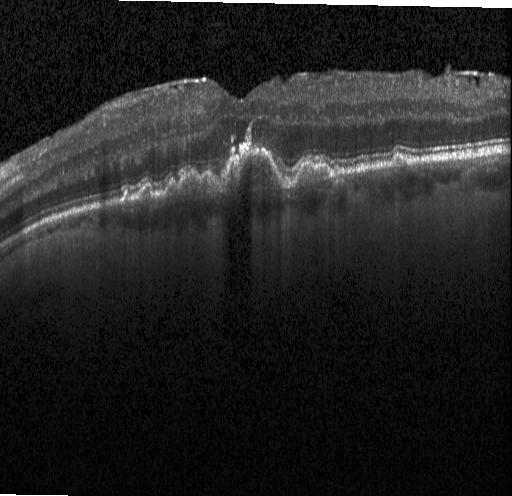

Spectral-domain OCT, optical coherence tomography scan.
Assessment: drusen.